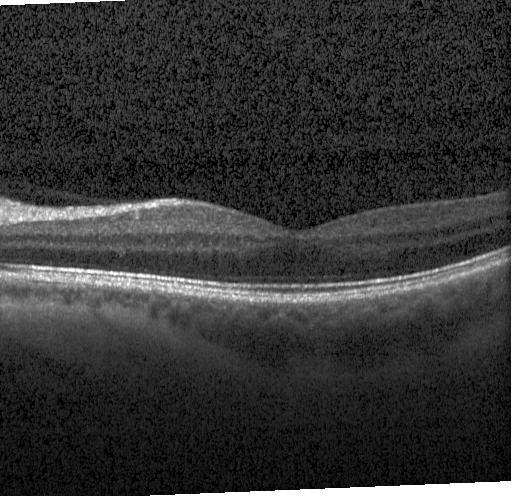 Heidelberg Spectralis. OCT B-scan. Horizontal scan through the fovea. Spectral-domain OCT. Impression: neither CNV, DME, nor drusen.